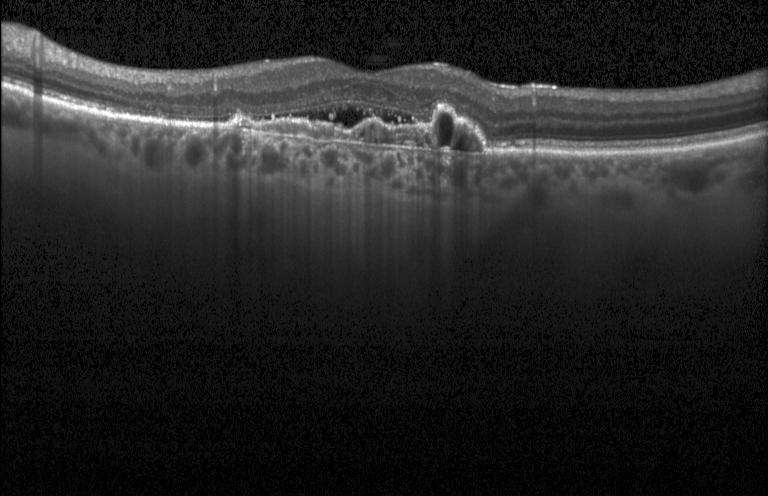
Macular OCT: a choroidal neovascular membrane.